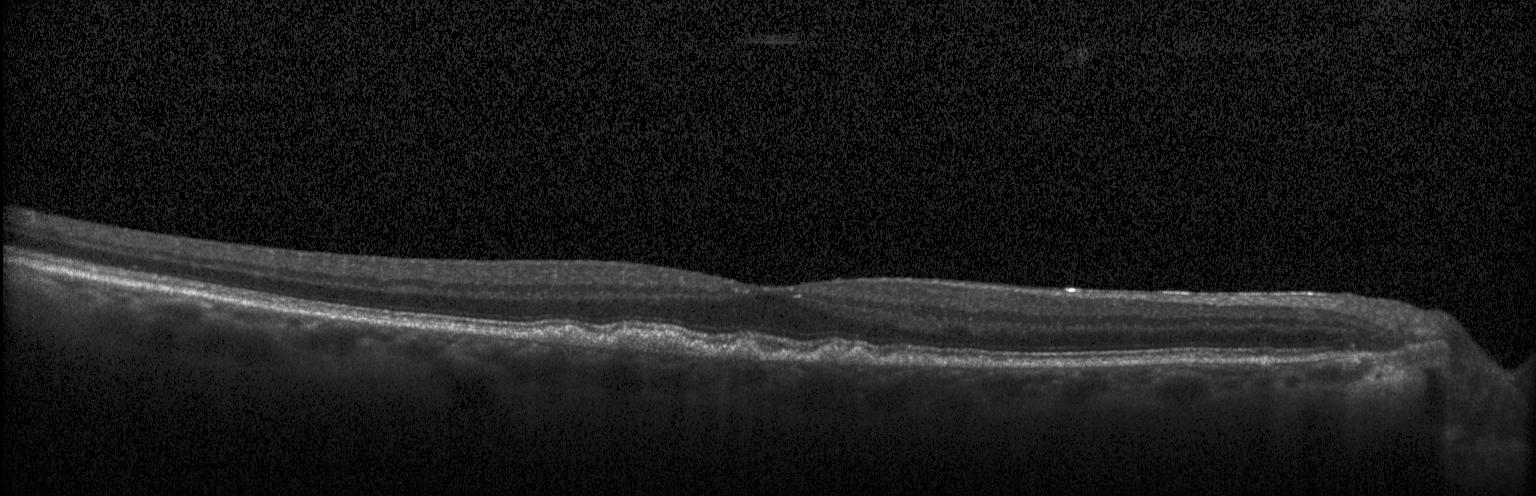 SD-OCT; Heidelberg Spectralis OCT system; retinal OCT B-scan; macular scan.
This B-scan demonstrates sub-RPE drusenoid deposits.